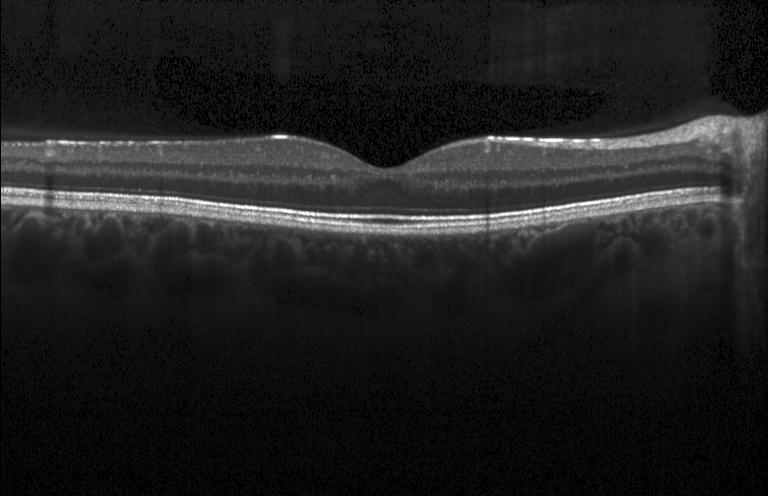
OCT B-scan — Finding: neither choroidal neovascularization, diabetic macular edema, nor drusen.